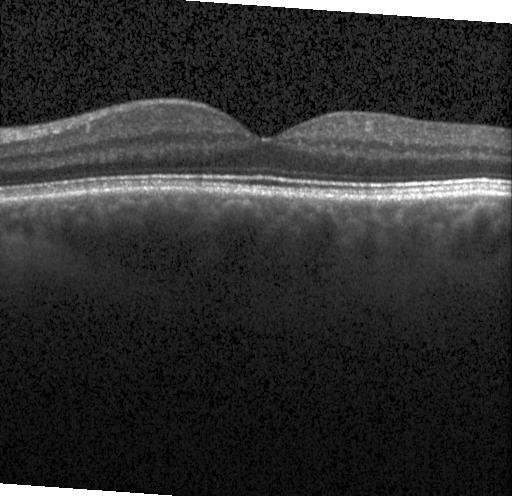

No CNV, DME, or drusen.